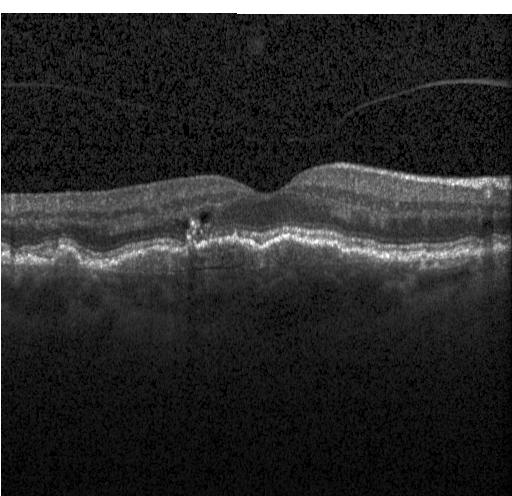 Retinal OCT B-scan, centered on the fovea, SD-OCT, Heidelberg Spectralis OCT system. Assessment: a choroidal neovascular membrane.